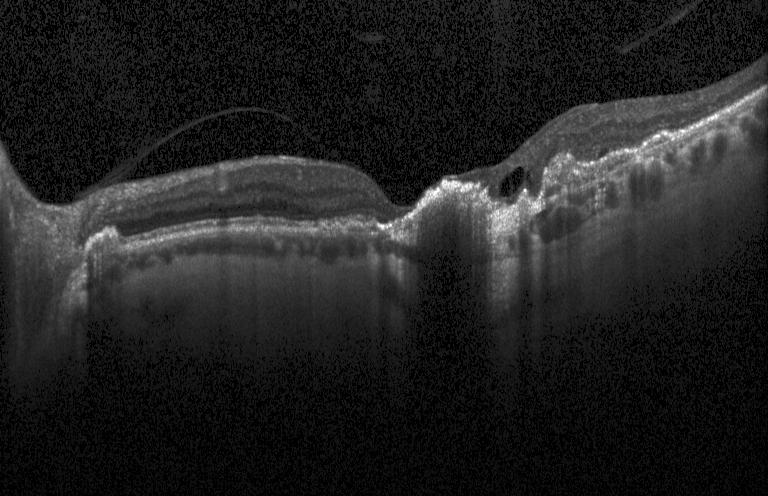 Retinal OCT B-scan.
Dx: a choroidal neovascular membrane.